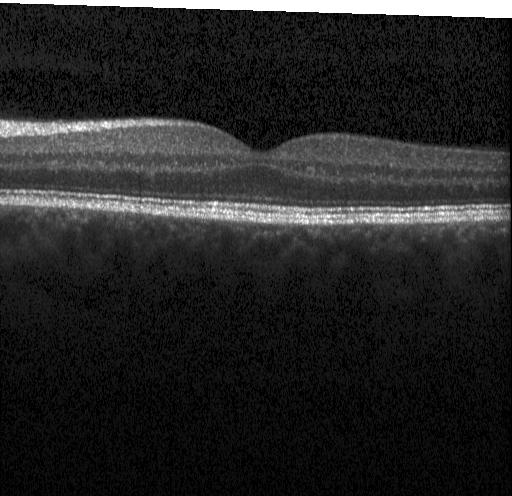

Macular OCT demonstrating no evidence of CNV, DME, or drusen.